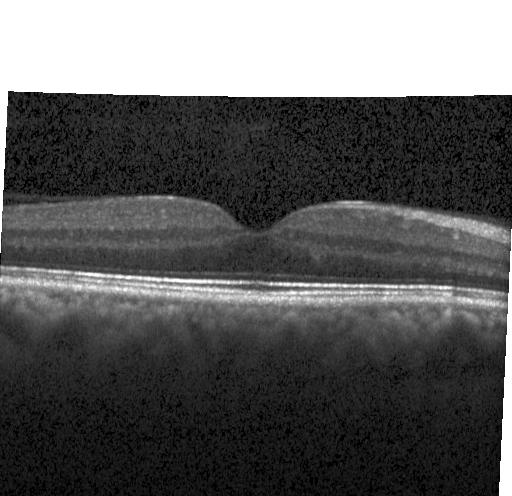

Spectral-domain optical coherence tomography · retinal OCT cross-section · centered on the fovea
Diagnosis: no CNV, DME, or drusen.